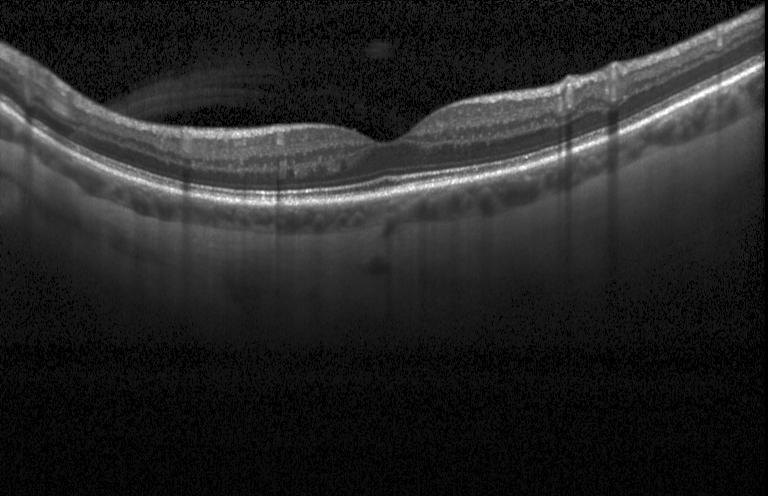

Instrument: Heidelberg Spectralis · OCT line scan · SD-OCT.
OCT finding: no choroidal neovascularization, no diabetic macular edema, and no drusen.